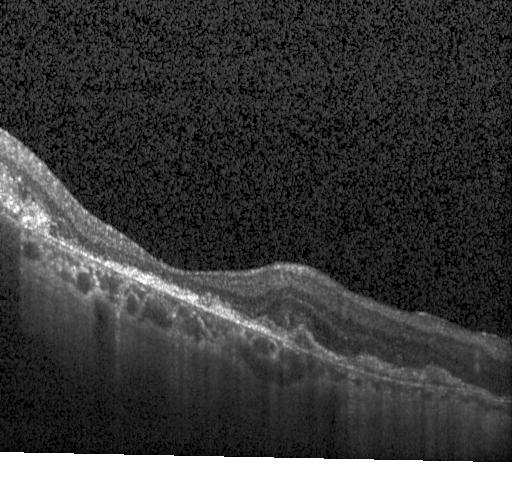 Macular scan. Retinal OCT cross-section. The scan shows a choroidal neovascular membrane.